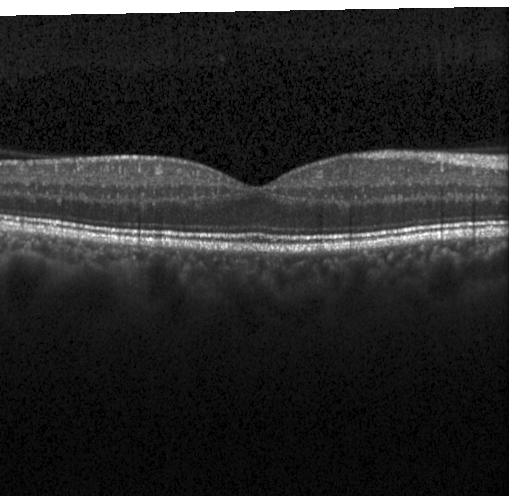

Spectral-domain OCT. Through the macula. Heidelberg Spectralis OCT system. Retinal OCT B-scan. No evidence of choroidal neovascularization, diabetic macular edema, or drusen.